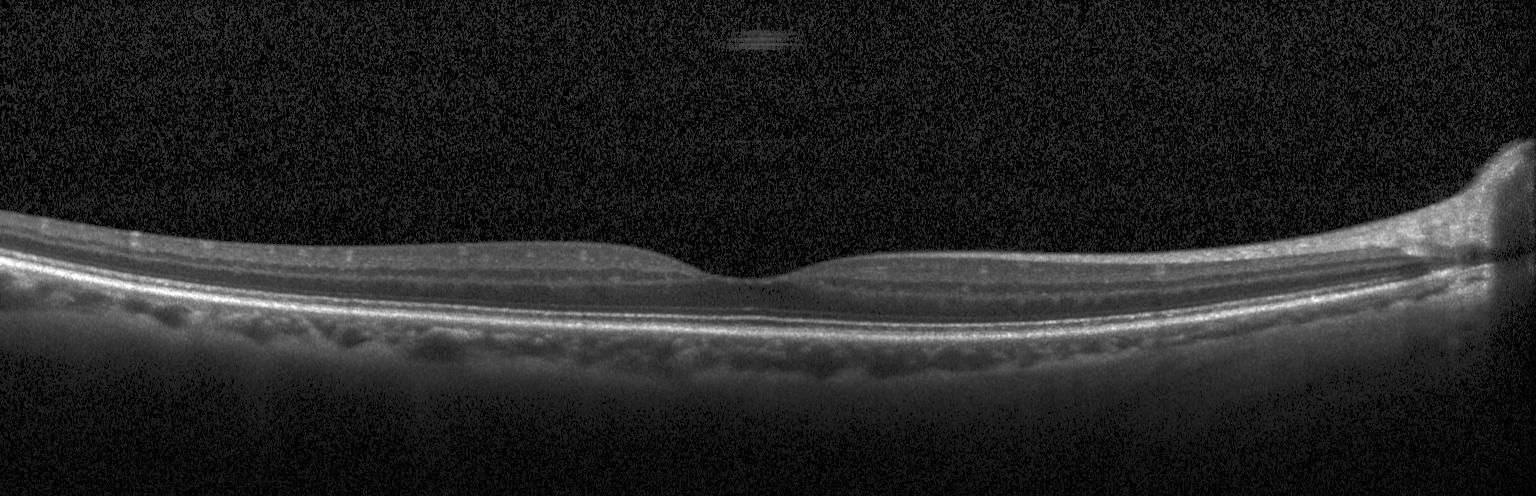 Dx: no choroidal neovascularization, diabetic macular edema, or drusen.